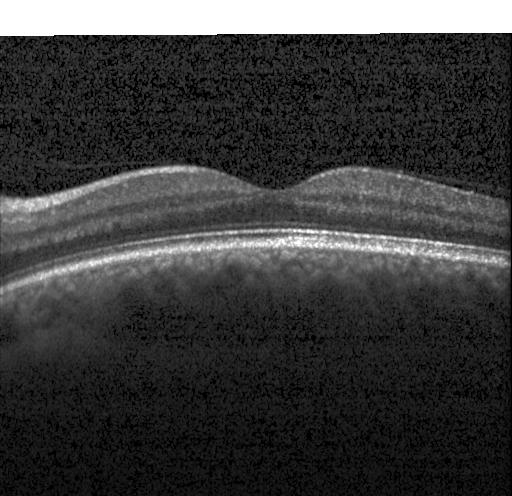
Acquired on a Heidelberg Spectralis, spectral-domain OCT, OCT B-scan. Assessment: no CNV, DME, or drusen.